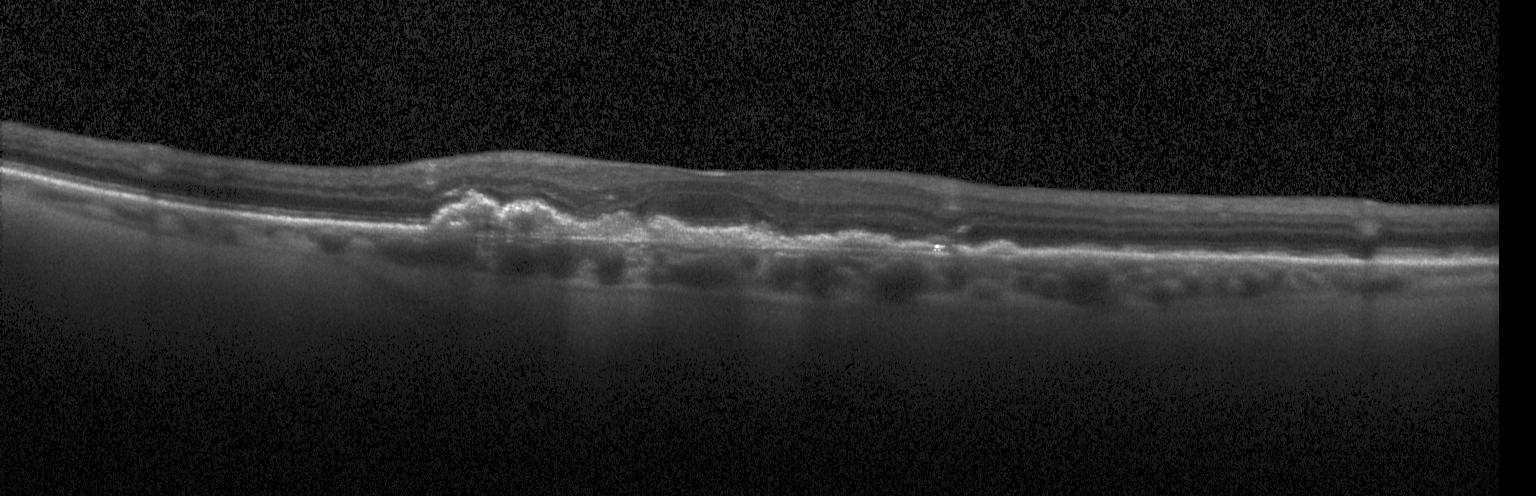 Finding: CNV.